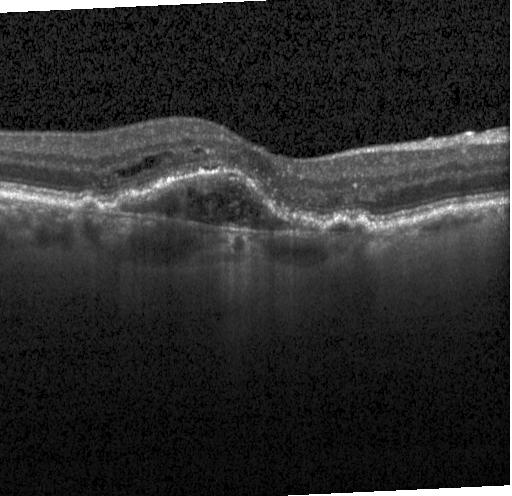 OCT B-scan; Heidelberg Spectralis OCT system; fovea-centered; SD-OCT
Impression: a choroidal neovascular membrane.